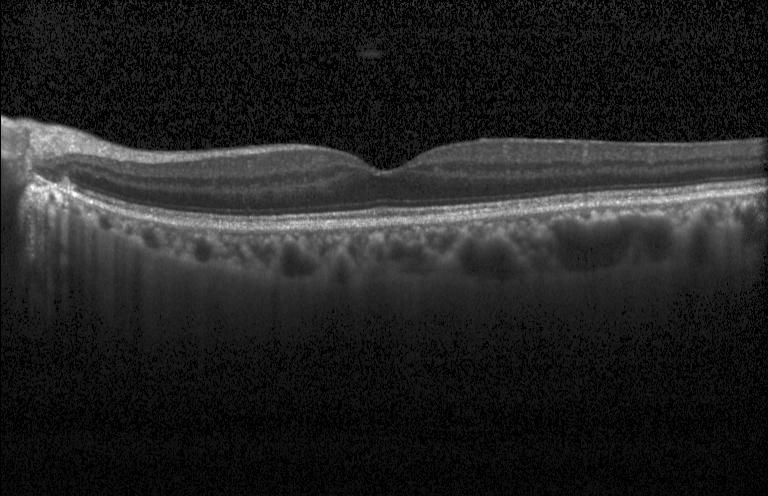
This B-scan demonstrates no choroidal neovascularization, diabetic macular edema, or drusen.